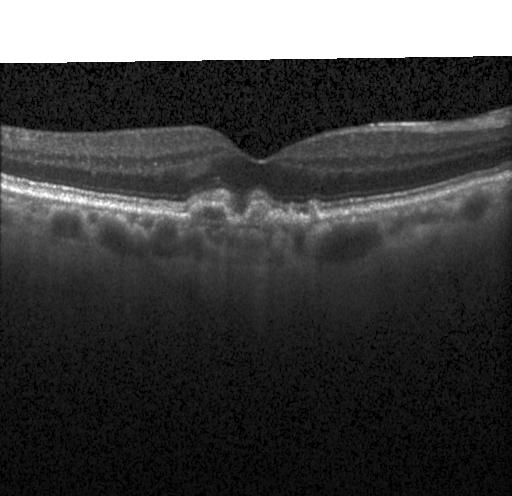

Finding: choroidal neovascularization (CNV).